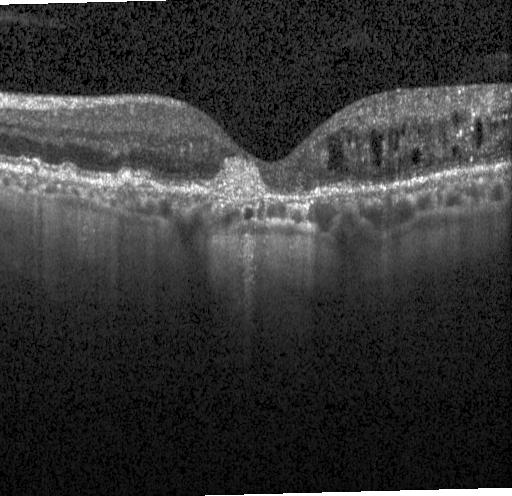

A choroidal neovascular membrane.